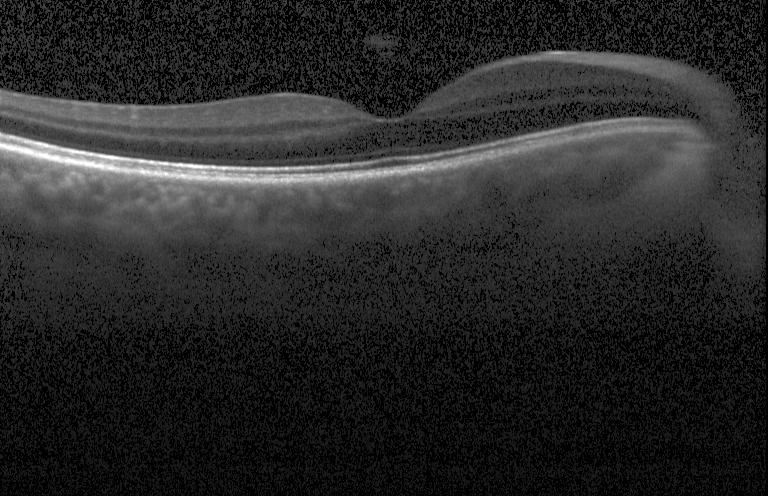 Heidelberg Spectralis OCT system. Spectral-domain optical coherence tomography. Retinal OCT B-scan — Diagnosis: no choroidal neovascularization, no diabetic macular edema, and no drusen.